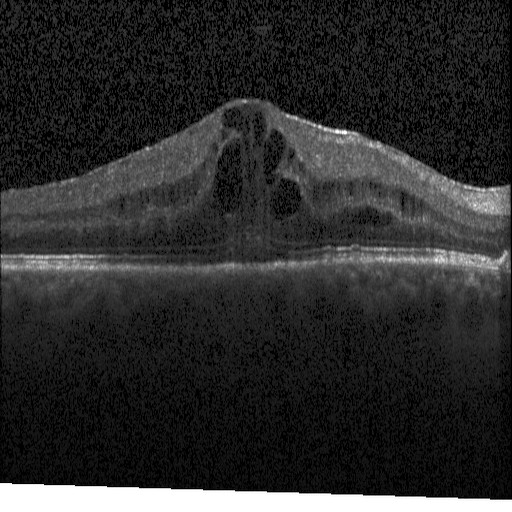

Retinal OCT B-scan; acquired on a Heidelberg Spectralis — Diagnosis: diabetic macular edema.